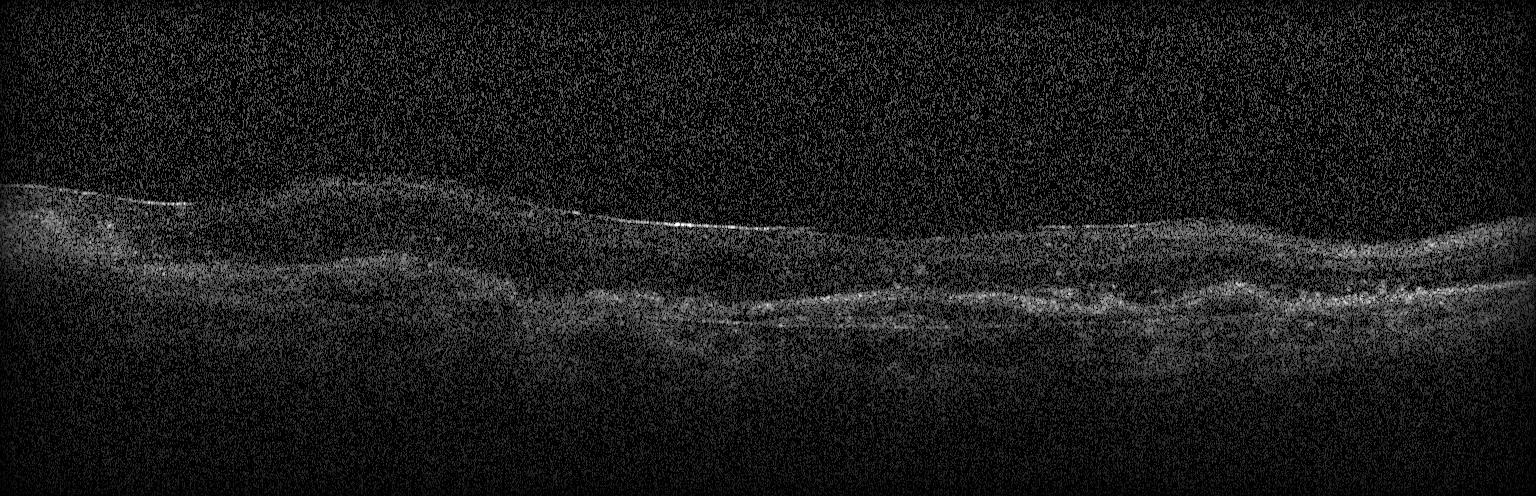
Retinal OCT B-scan, Heidelberg Spectralis OCT system, spectral-domain OCT, fovea-centered.
CNV.